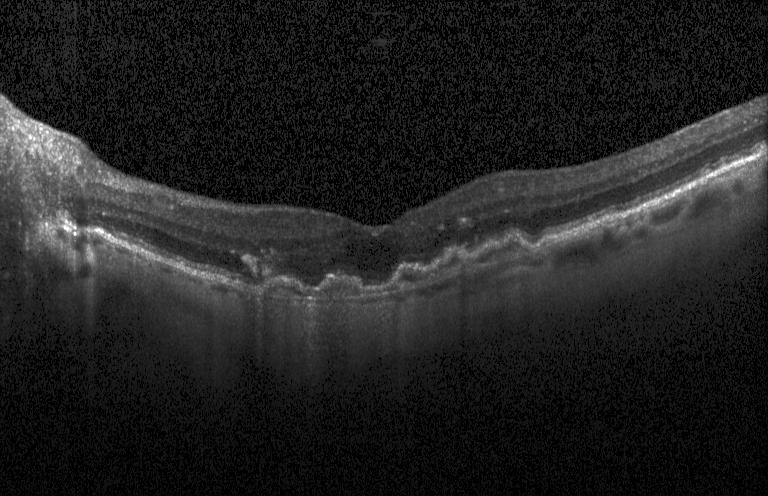

Through the macula, Heidelberg Spectralis OCT system, optical coherence tomography scan, spectral-domain optical coherence tomography. A choroidal neovascular membrane.